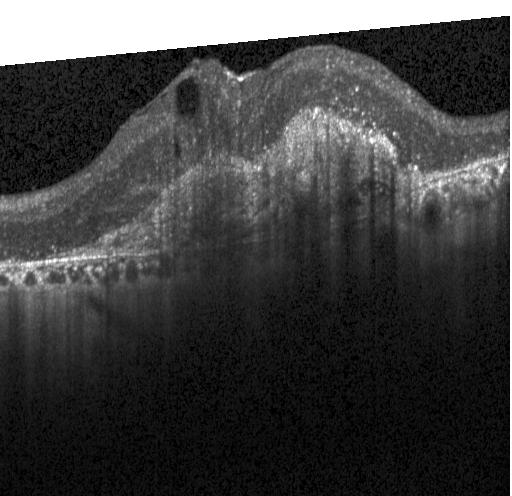
Diagnosis: choroidal neovascularization (CNV).